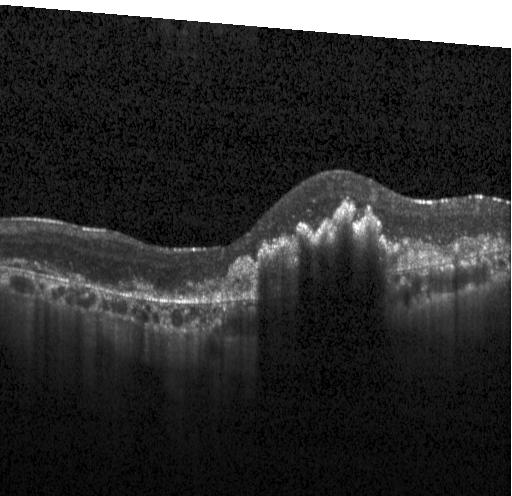
Spectral-domain OCT; Heidelberg Spectralis; retinal OCT B-scan — Finding: choroidal neovascularization (CNV).